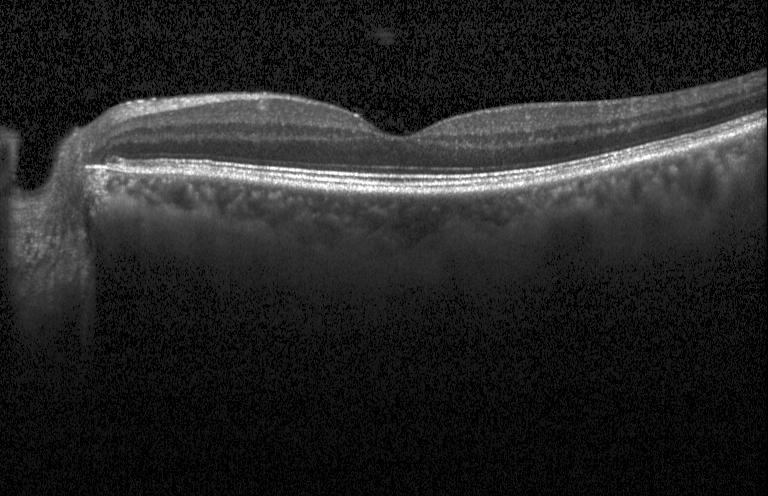
Instrument: Heidelberg Spectralis; macular scan; spectral-domain OCT; OCT B-scan.
Dx: no choroidal neovascularization, no diabetic macular edema, and no drusen.